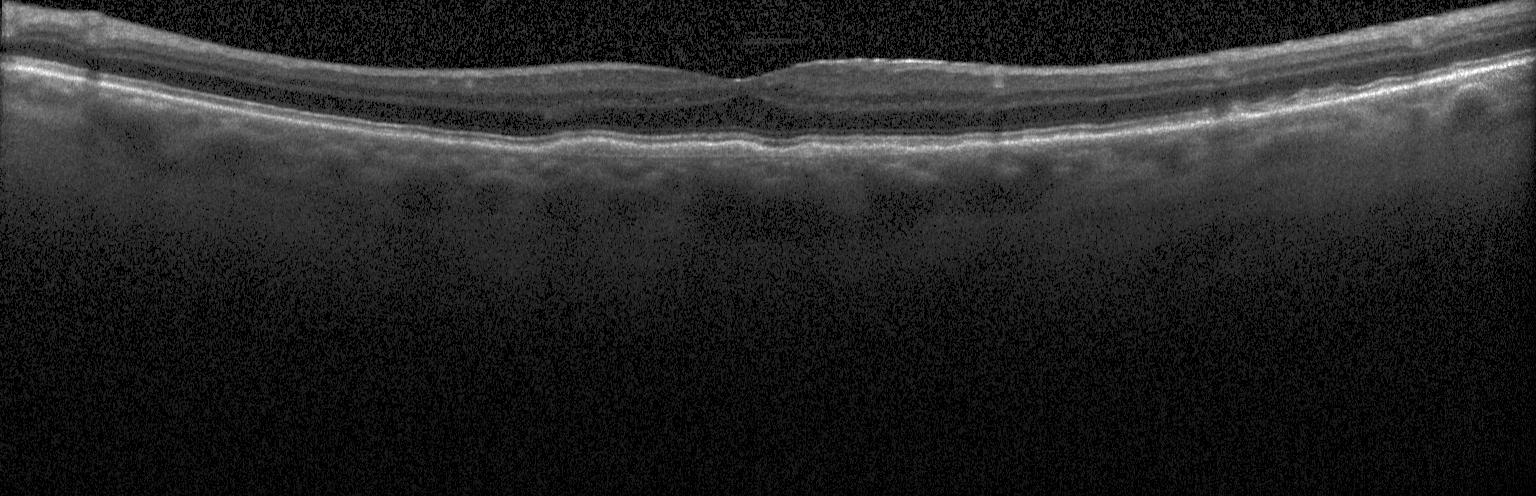 Macular OCT: a choroidal neovascular membrane.